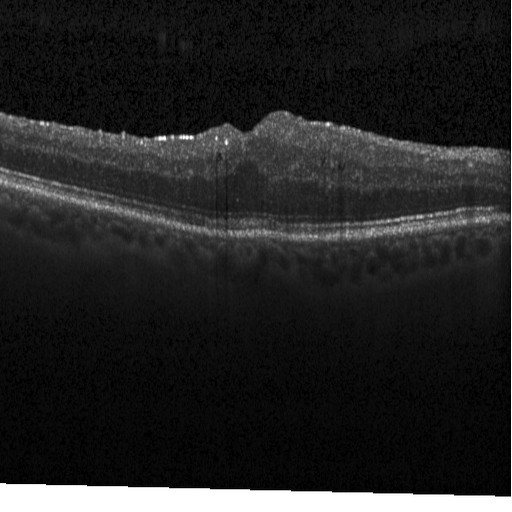
OCT B-scan, fovea-centered, SD-OCT. Diagnosis: diabetic macular edema (DME).